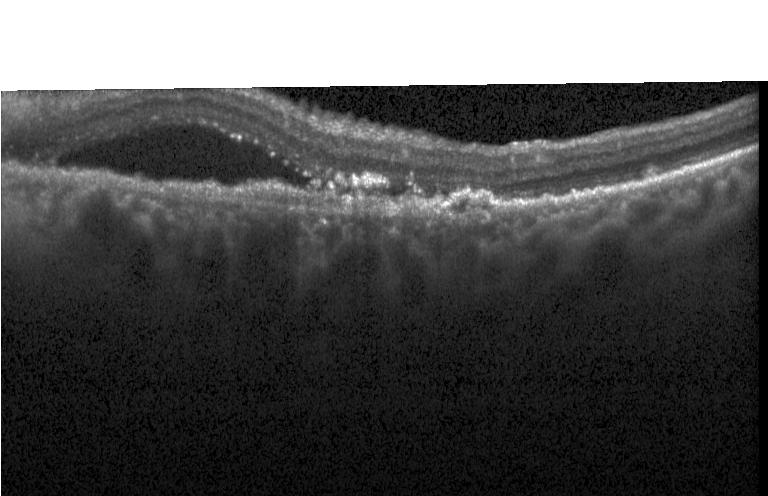 Retinal OCT B-scan. Horizontal scan through the fovea. Spectral-domain optical coherence tomography. Diagnosis: a choroidal neovascular membrane.